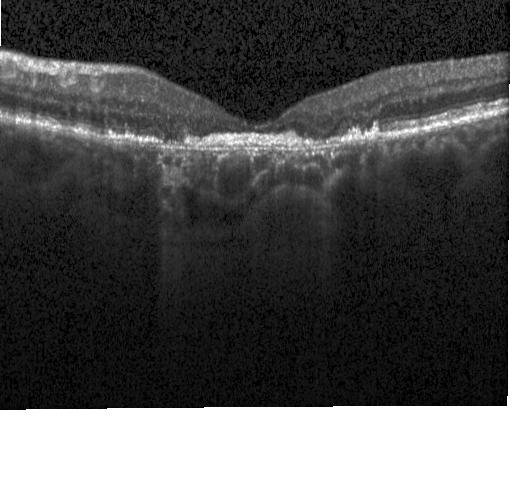 Retinal OCT cross-section. Heidelberg Spectralis OCT system — Finding: CNV.